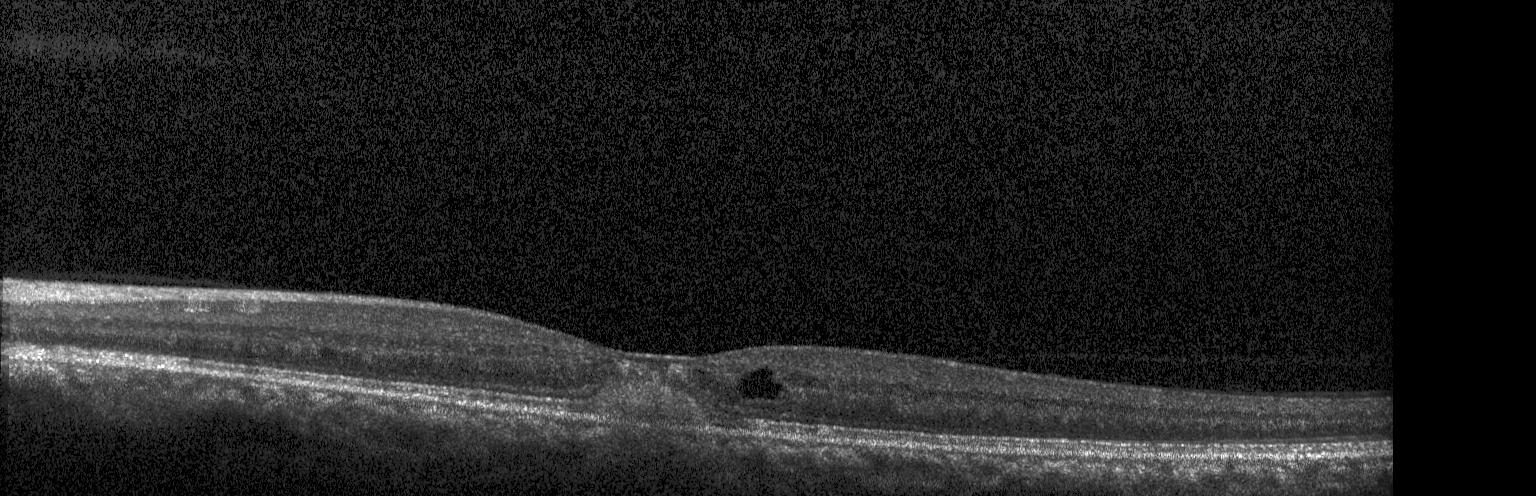

Heidelberg Spectralis OCT system; retinal OCT B-scan; horizontal scan through the fovea; spectral-domain OCT.
Assessment: a choroidal neovascular membrane.